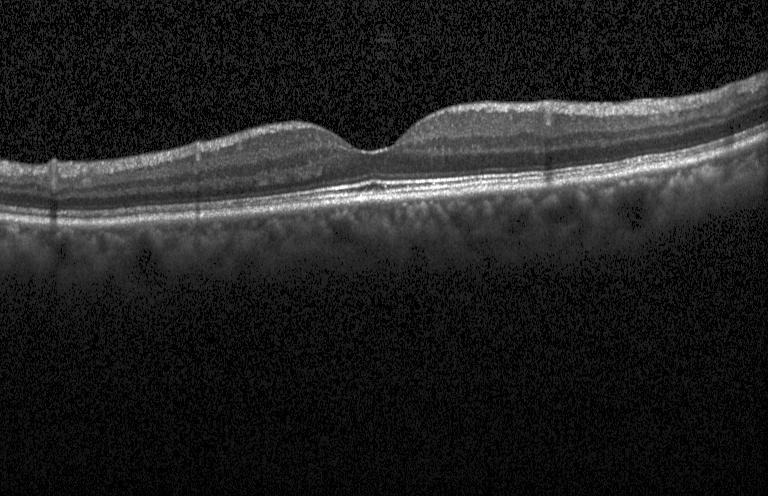 Heidelberg Spectralis OCT system · OCT line scan · spectral-domain OCT · centered on the fovea
Diagnosis: no choroidal neovascularization, diabetic macular edema, or drusen.